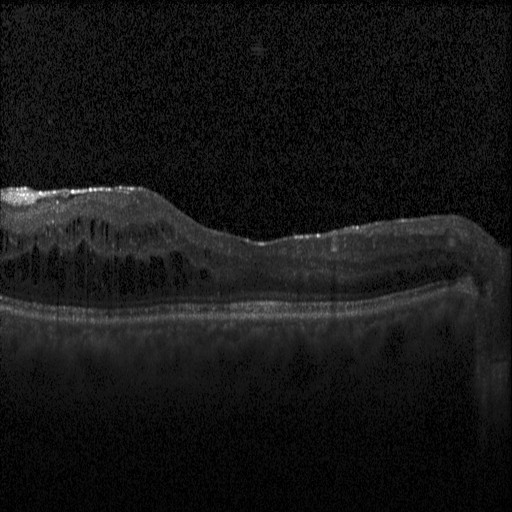 Optical coherence tomography scan · Heidelberg Spectralis · spectral-domain OCT. Macular OCT: diabetic macular edema.